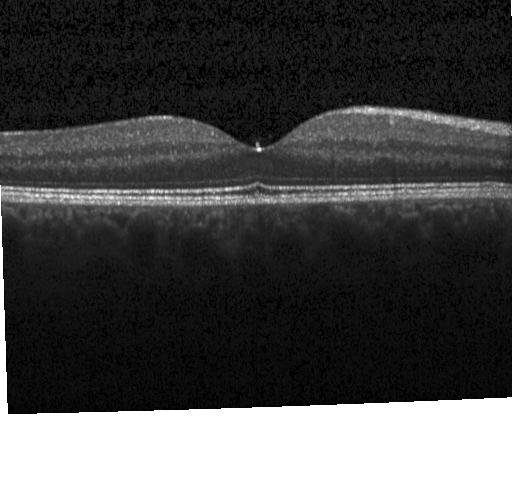

SD-OCT. OCT B-scan.
Diagnosis: no choroidal neovascularization, no diabetic macular edema, and no drusen.